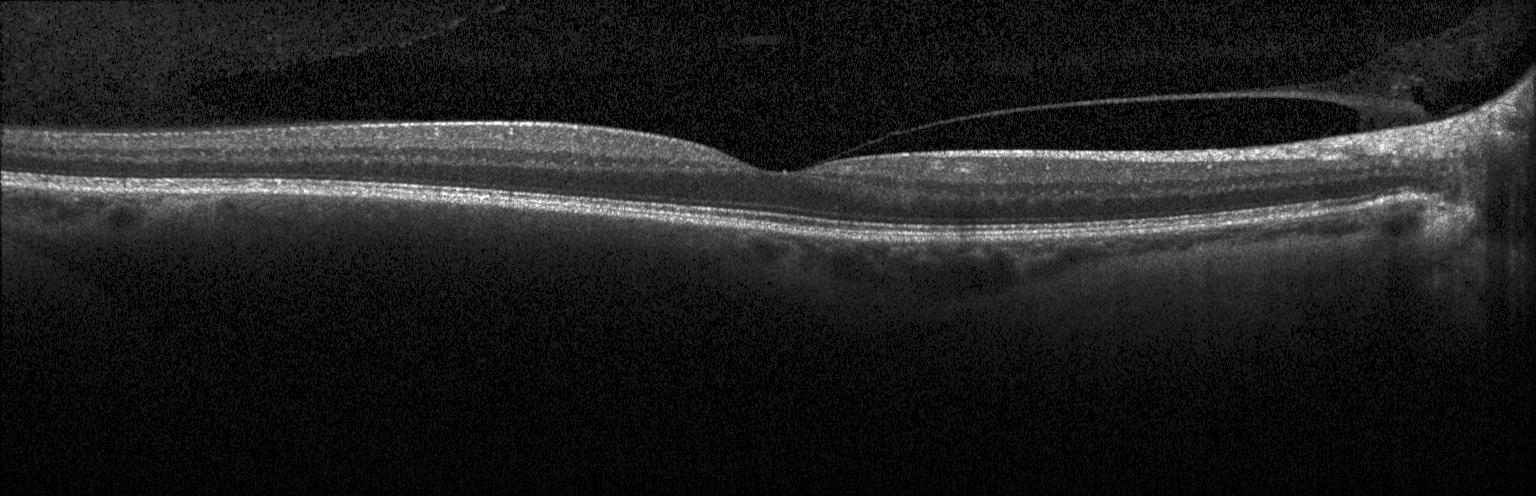 OCT B-scan showing no evidence of choroidal neovascularization, diabetic macular edema, or drusen.